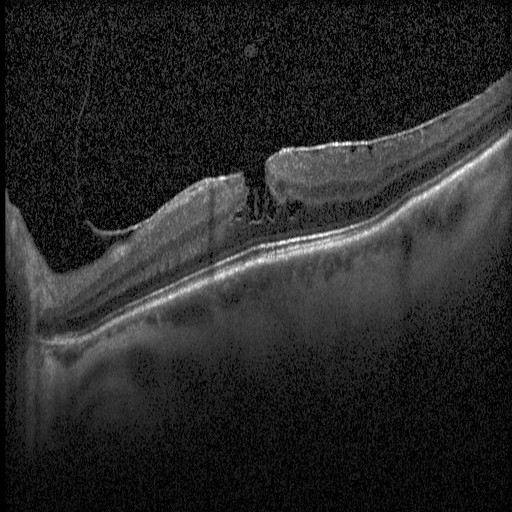 Impression: diabetic macular edema (DME).